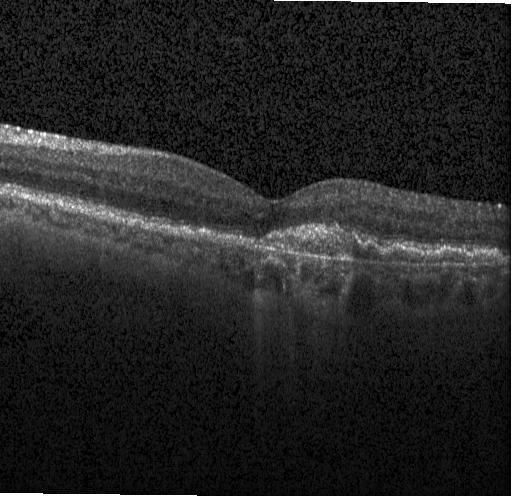

OCT B-scan · SD-OCT · acquired on a Heidelberg Spectralis · fovea-centered.
Impression: CNV.